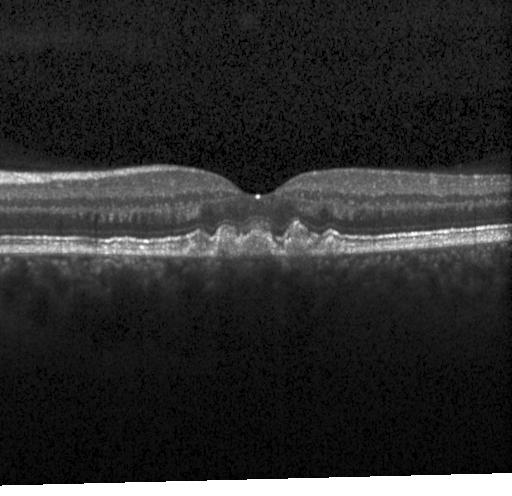

Optical coherence tomography scan.
Diagnosis: drusen.